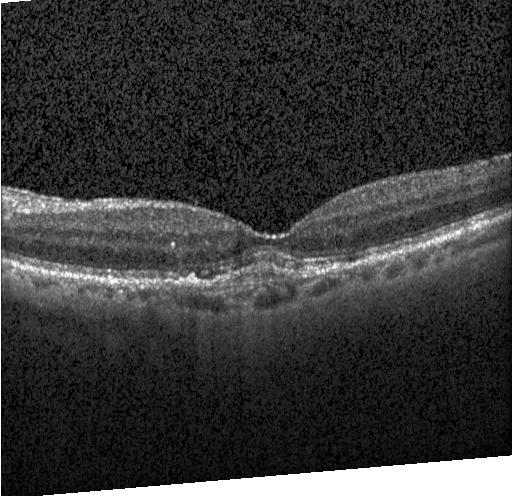

The scan shows CNV.